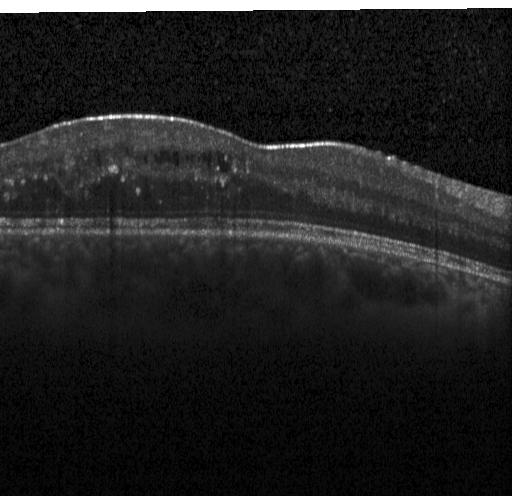
Diagnosis: diabetic macular edema (DME).